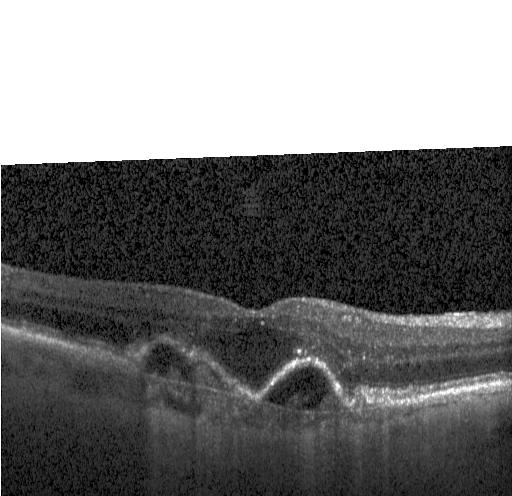
OCT finding: CNV.